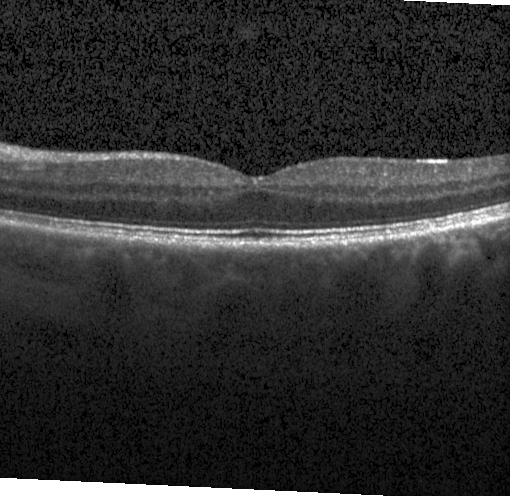

Optical coherence tomography B-scan · SD-OCT — Assessment: no evidence of CNV, DME, or drusen.